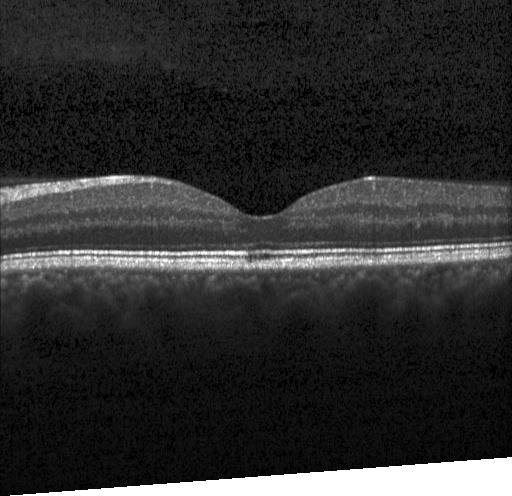
Heidelberg Spectralis OCT system. Optical coherence tomography scan. SD-OCT. Macular OCT: no choroidal neovascularization, diabetic macular edema, or drusen.